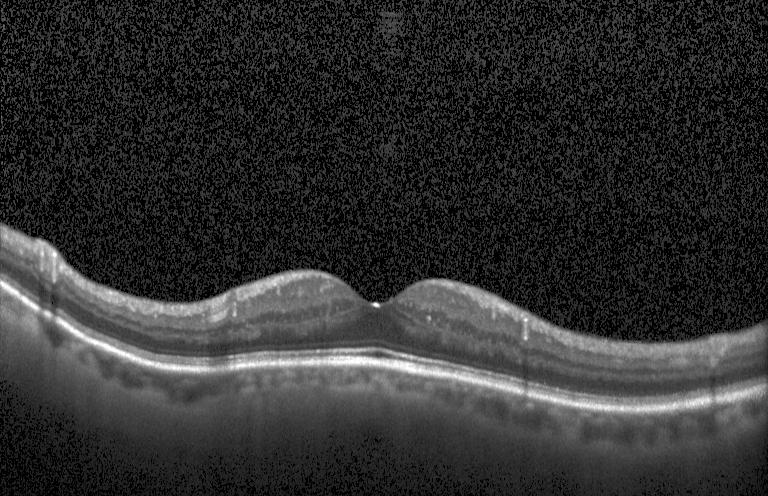
The scan shows no evidence of choroidal neovascularization, diabetic macular edema, or drusen.